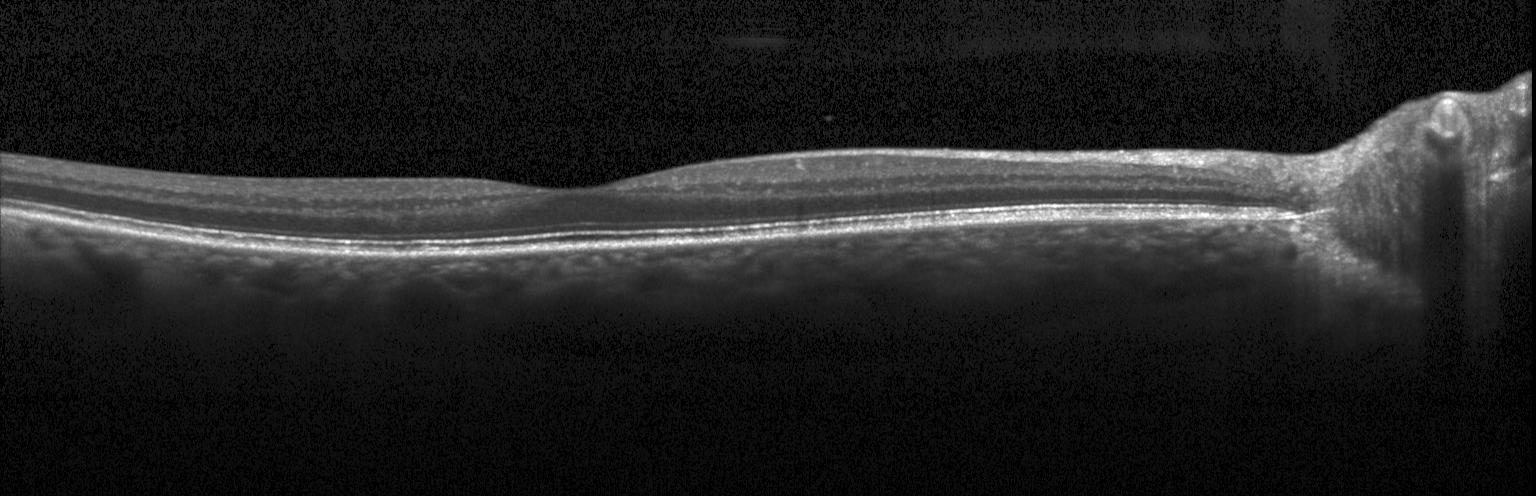

The scan shows neither choroidal neovascularization, diabetic macular edema, nor drusen.